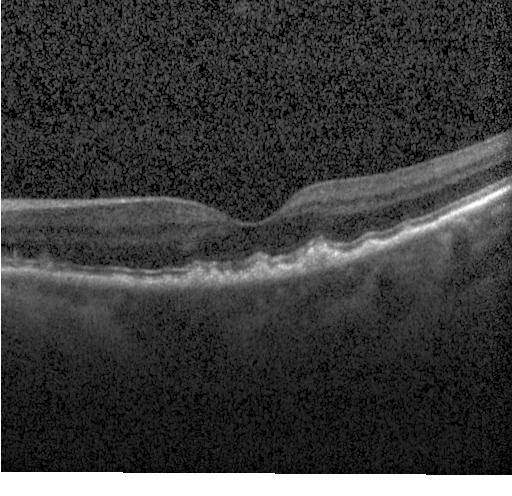 Finding: multiple drusen.